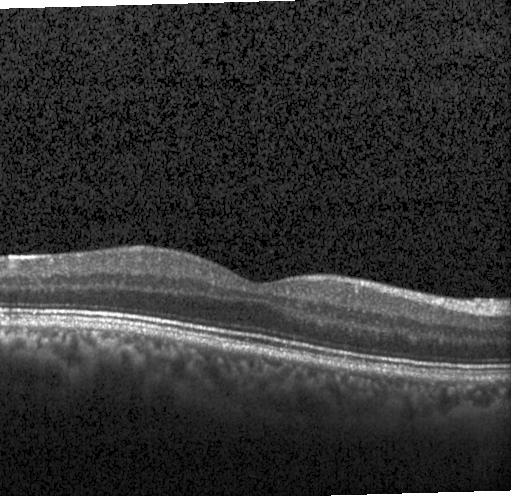 Macular OCT: no choroidal neovascularization, diabetic macular edema, or drusen.